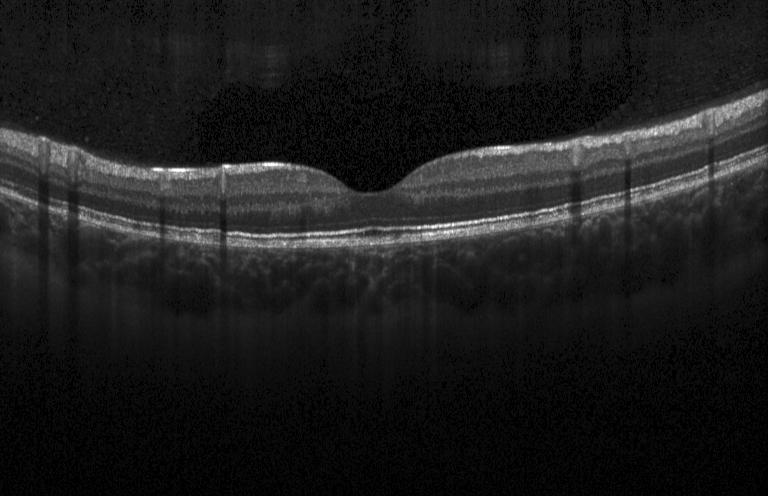
Retinal OCT cross-section, acquired on a Heidelberg Spectralis. Neither choroidal neovascularization, diabetic macular edema, nor drusen.